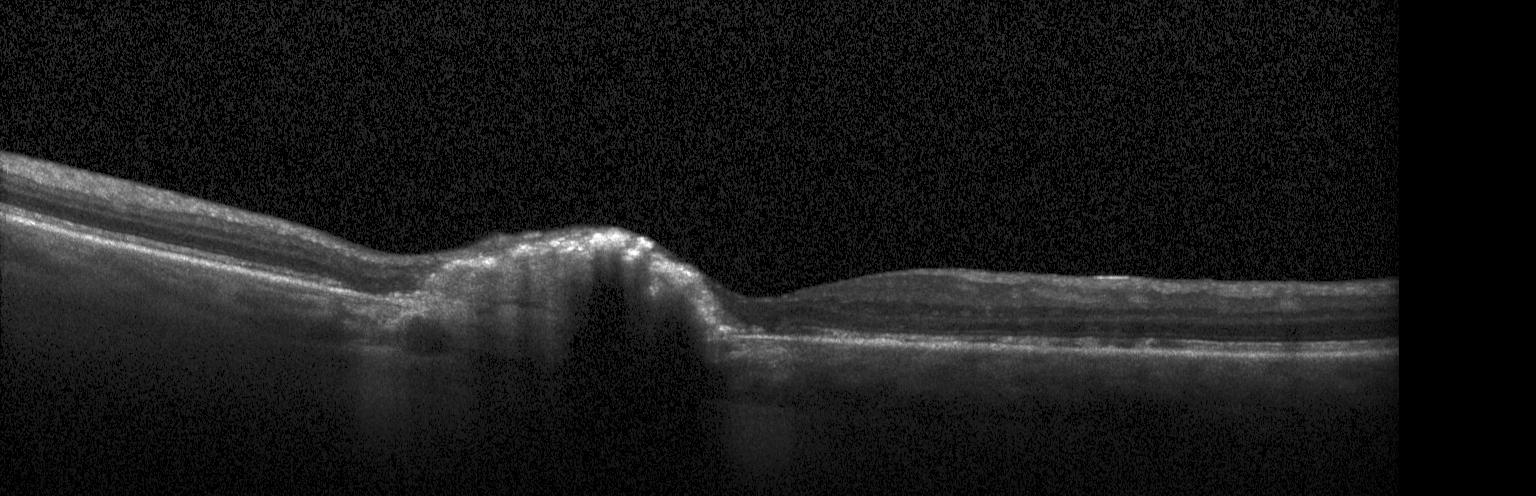

Optical coherence tomography B-scan — Macular OCT: a choroidal neovascular membrane.